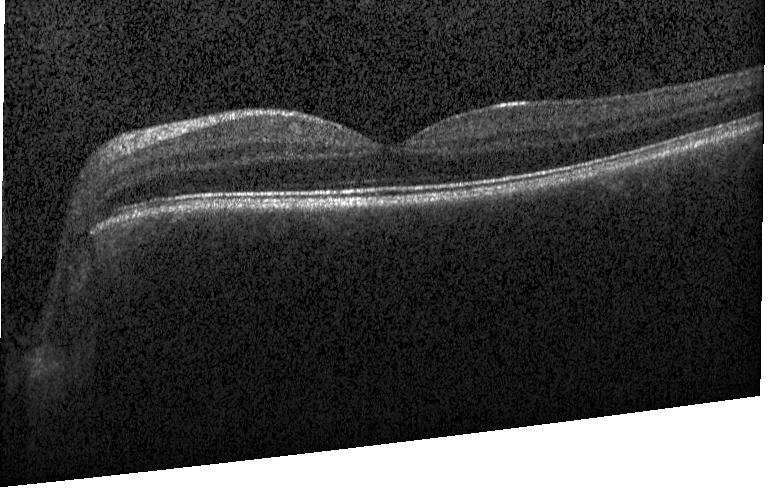

OCT line scan · macular scan · instrument: Heidelberg Spectralis · spectral-domain optical coherence tomography — Diagnosis: no choroidal neovascularization, no diabetic macular edema, and no drusen.